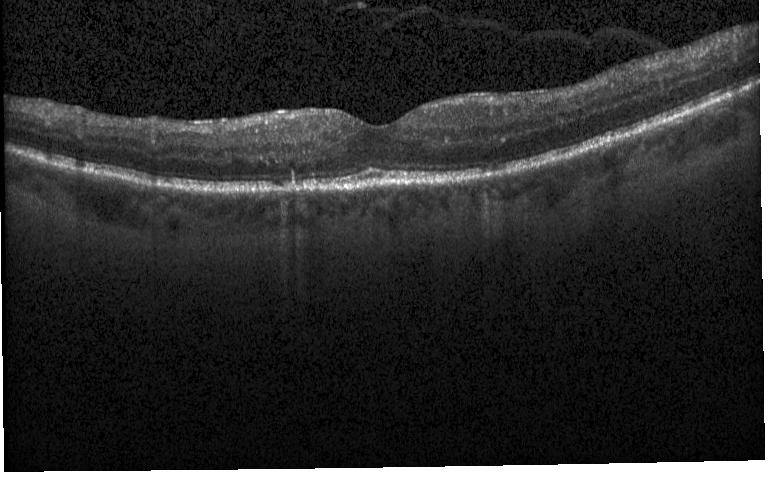

Spectral-domain OCT B-scan: DME.